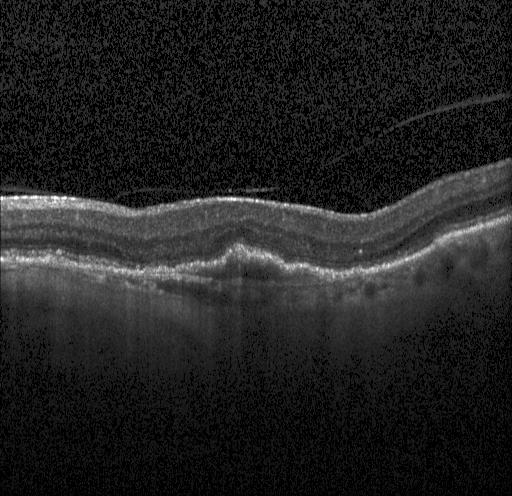 Spectral-domain optical coherence tomography. Macular scan. Optical coherence tomography B-scan. The scan shows a choroidal neovascular membrane.